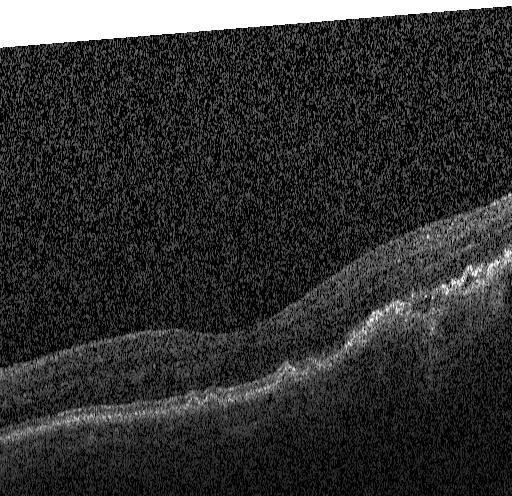
The scan shows a choroidal neovascular membrane.